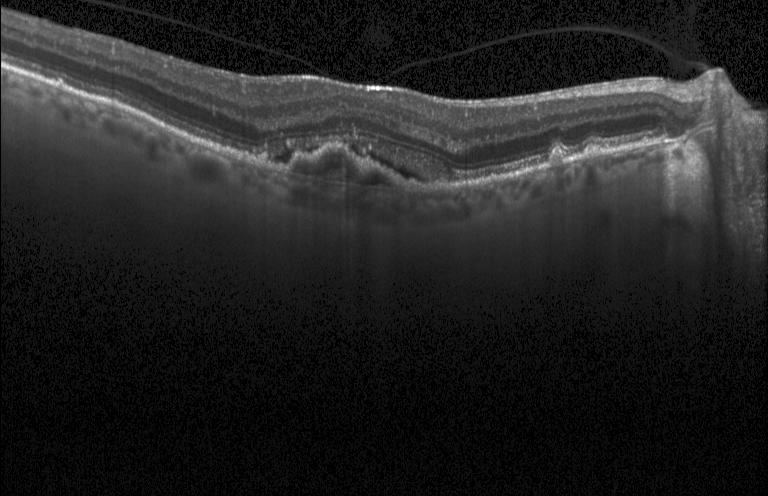 Fovea-centered; optical coherence tomography scan; Heidelberg Spectralis; spectral-domain optical coherence tomography. Impression: a choroidal neovascular membrane.